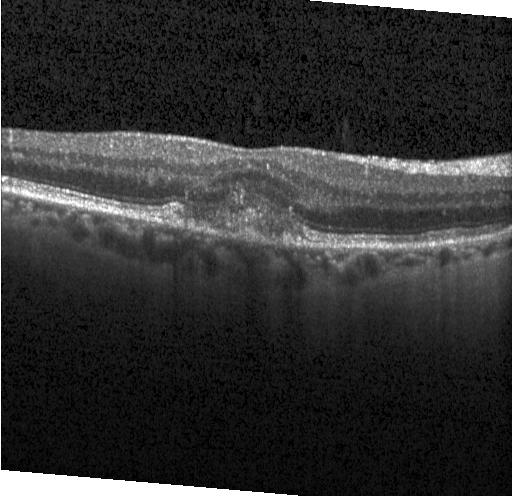

Heidelberg Spectralis OCT system; OCT line scan; centered on the fovea; spectral-domain optical coherence tomography — Assessment: a choroidal neovascular membrane.